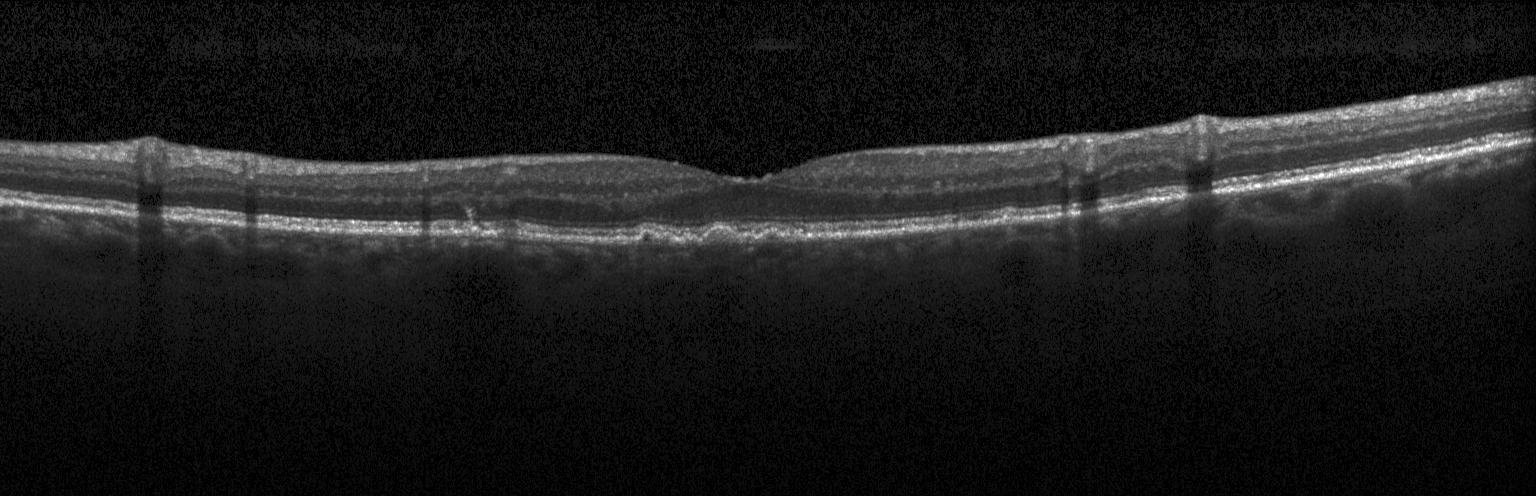
Fovea-centered · instrument: Heidelberg Spectralis · OCT B-scan
Drusen.